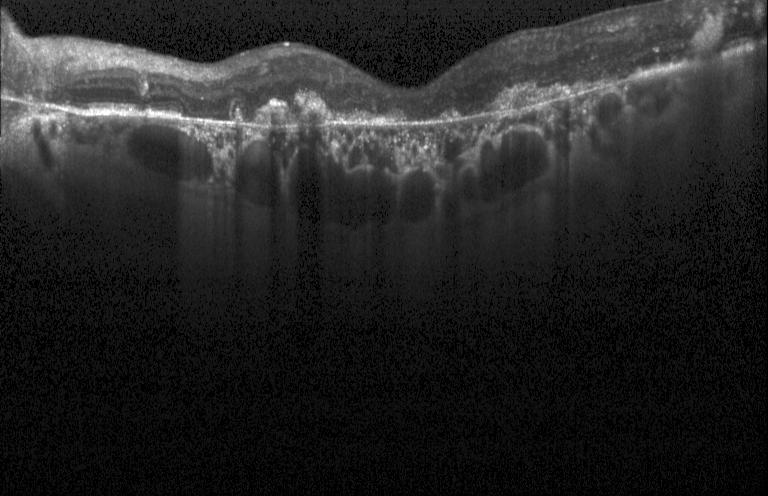

Heidelberg Spectralis; OCT B-scan; through the macula; spectral-domain optical coherence tomography
Assessment: a choroidal neovascular membrane.